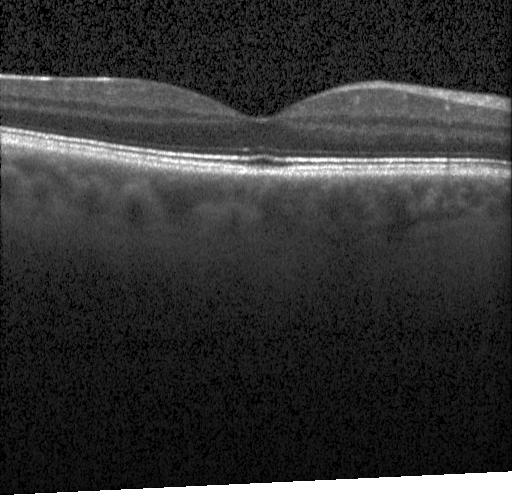
Macular scan. Spectral-domain OCT. OCT line scan. Acquired on a Heidelberg Spectralis — OCT finding: no choroidal neovascularization, no diabetic macular edema, and no drusen.